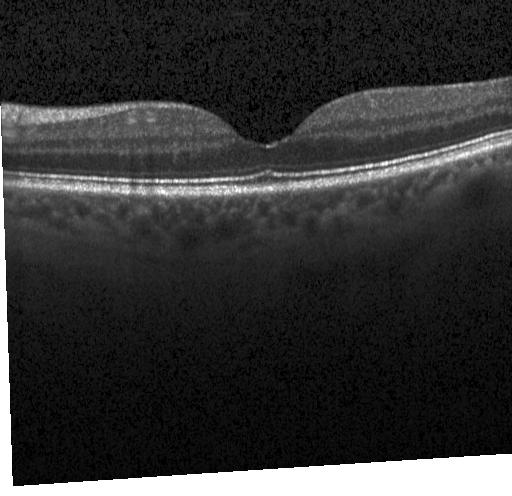

Spectral-domain OCT. OCT line scan
Assessment: no choroidal neovascularization, diabetic macular edema, or drusen.